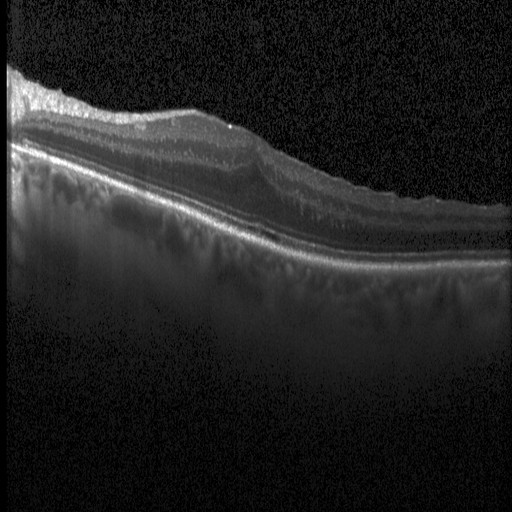 Finding: DME.